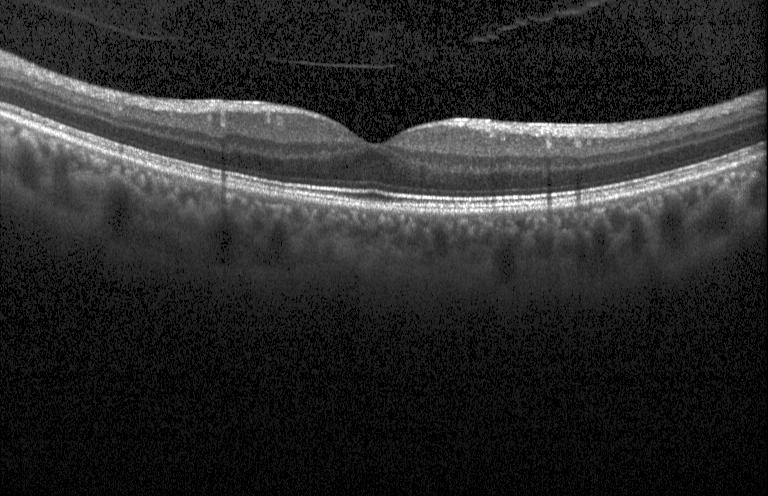
Retinal OCT B-scan · spectral-domain OCT · horizontal scan through the fovea · Heidelberg Spectralis OCT system. No CNV, no DME, and no drusen.